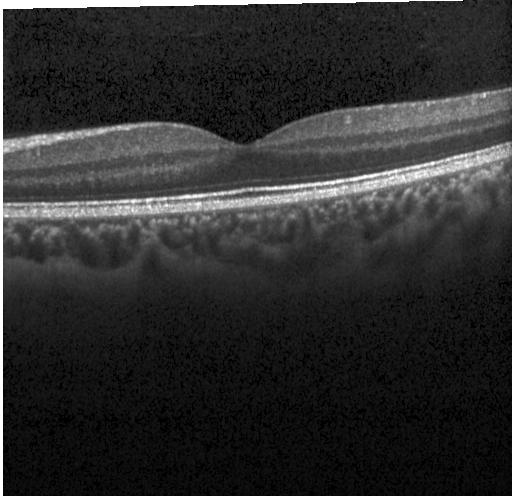 OCT line scan.
No CNV, no DME, and no drusen.